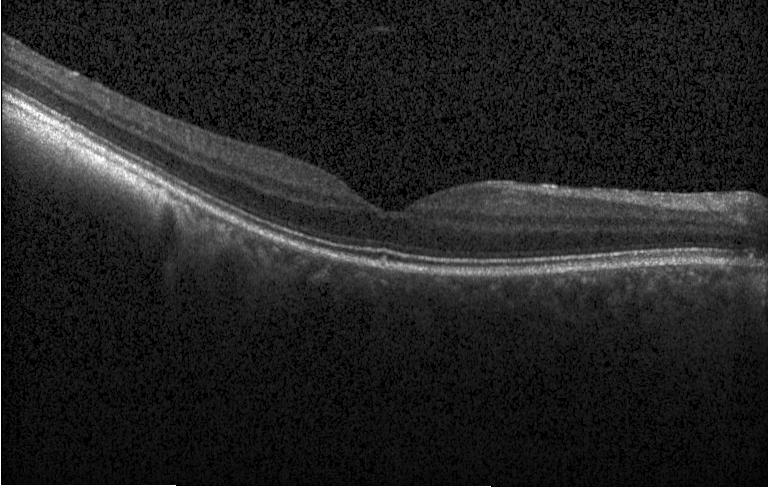

Retinal OCT cross-section showing multiple drusen.